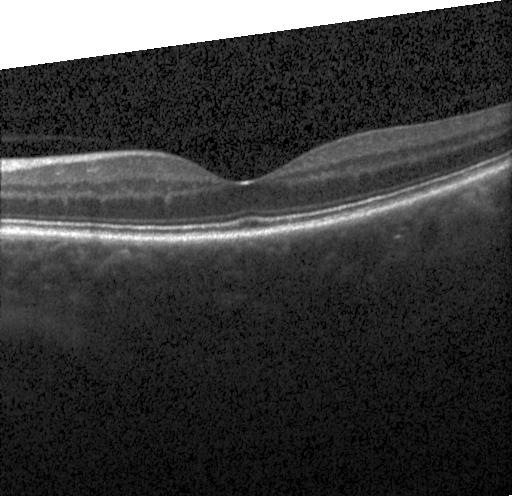
Macular scan. Heidelberg Spectralis. OCT line scan.
Macular OCT: no evidence of CNV, DME, or drusen.